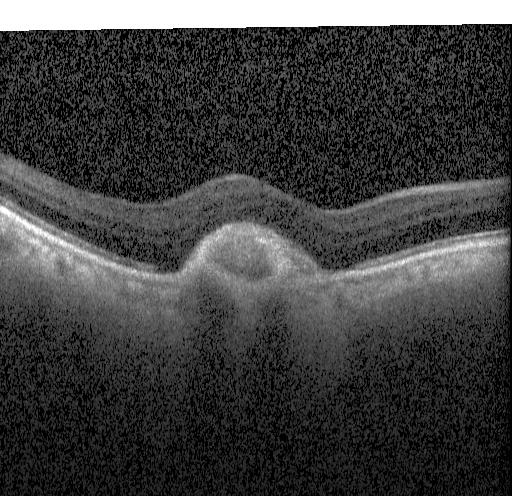

Impression: a choroidal neovascular membrane.